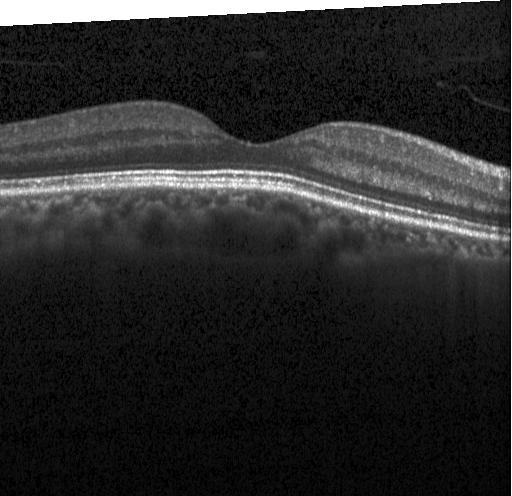

OCT line scan, instrument: Heidelberg Spectralis, spectral-domain OCT
OCT finding: no choroidal neovascularization, diabetic macular edema, or drusen.